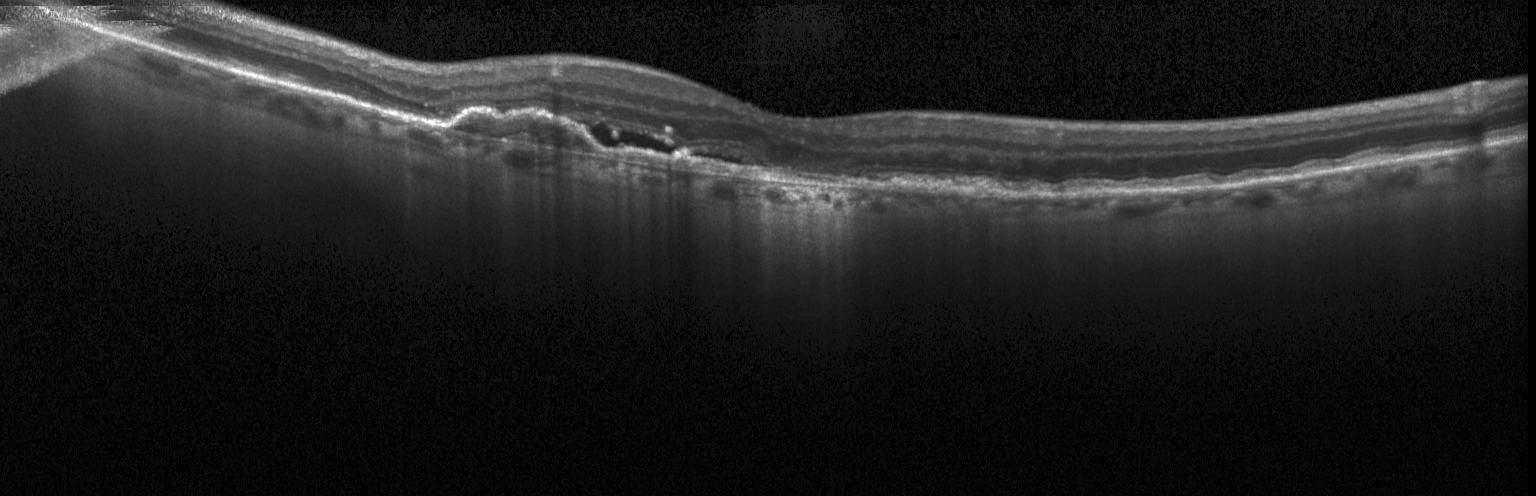
Macular OCT: choroidal neovascularization (CNV).